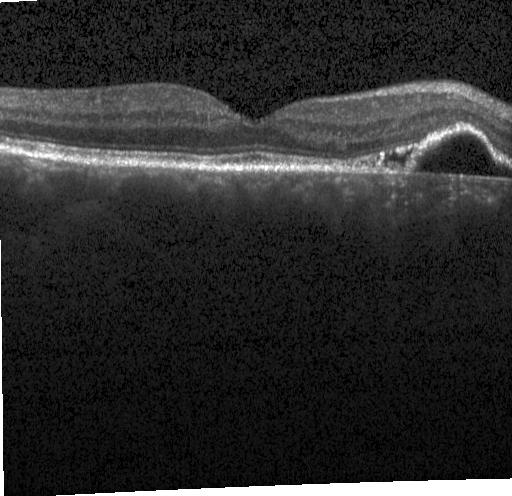

OCT B-scan; instrument: Heidelberg Spectralis — Impression: a choroidal neovascular membrane.